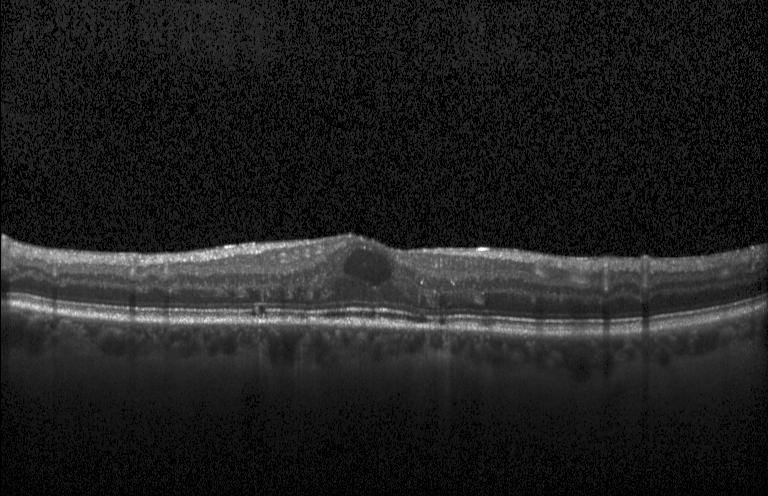

Assessment: diabetic macular edema.